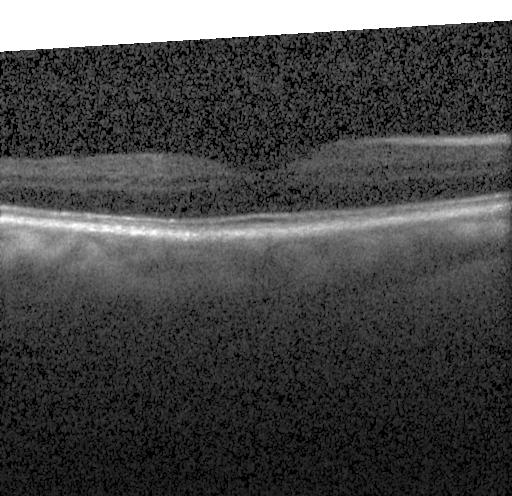

OCT scan showing no CNV, DME, or drusen.